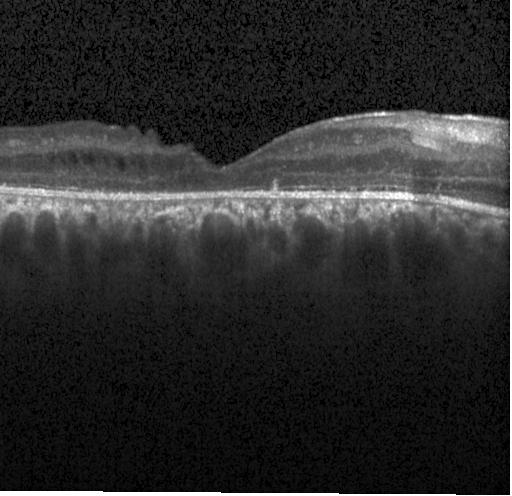

Retinal OCT cross-section — Impression: diabetic macular edema.